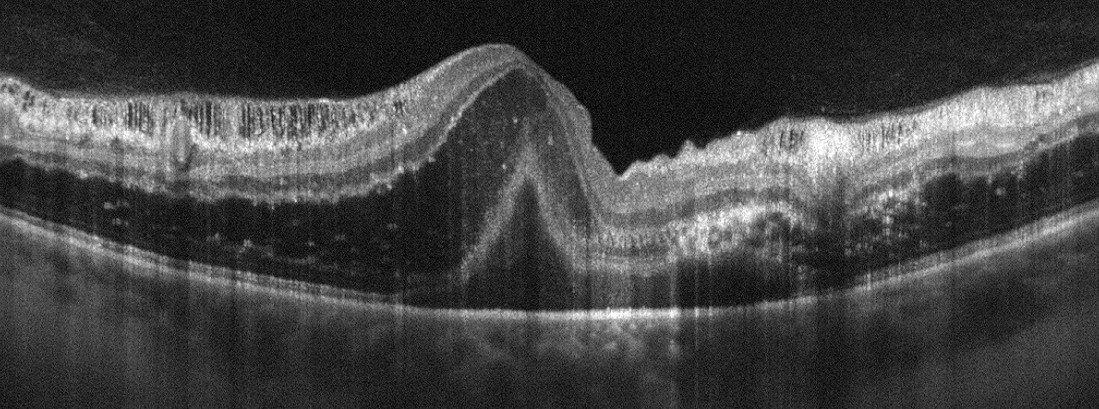
Instrument: Optovue Avanti RTVue XR, fovea-centered, optical coherence tomography B-scan
This B-scan demonstrates RVO.